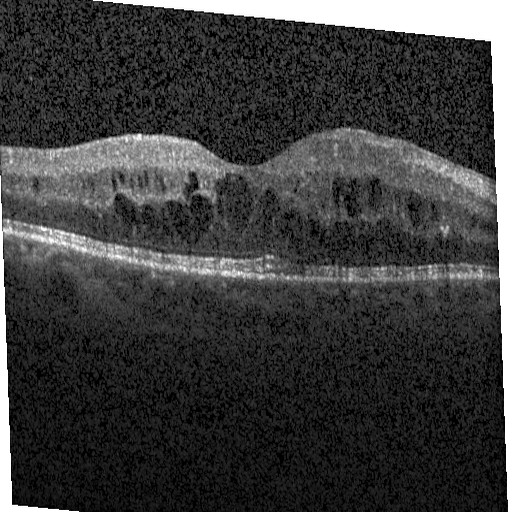

Dx: diabetic macular edema.